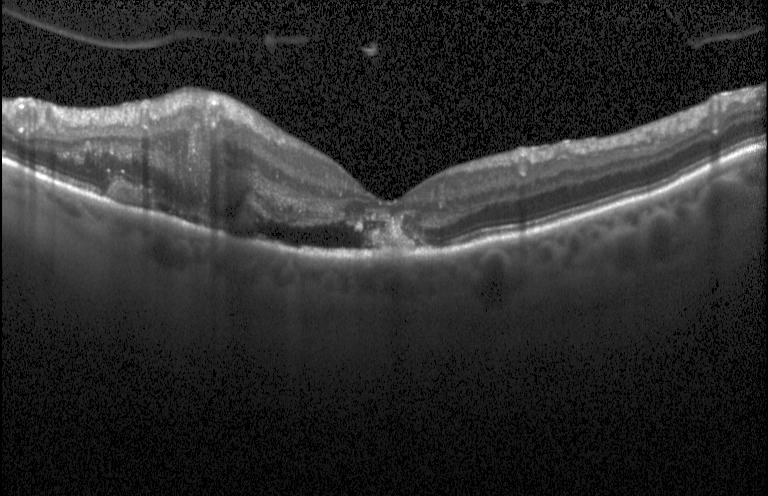

Spectral-domain OCT, Heidelberg Spectralis, macular scan, optical coherence tomography scan. Finding: CNV.